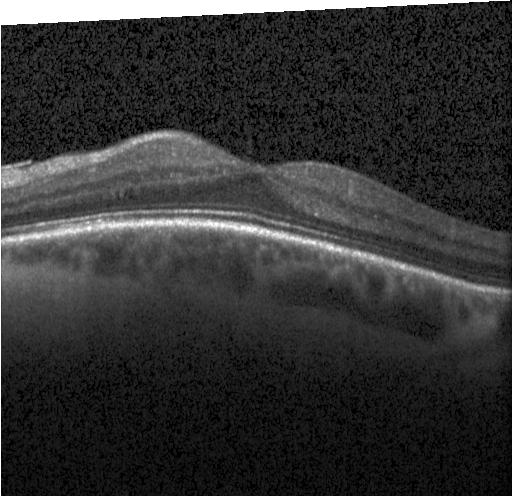 OCT finding: neither choroidal neovascularization, diabetic macular edema, nor drusen.